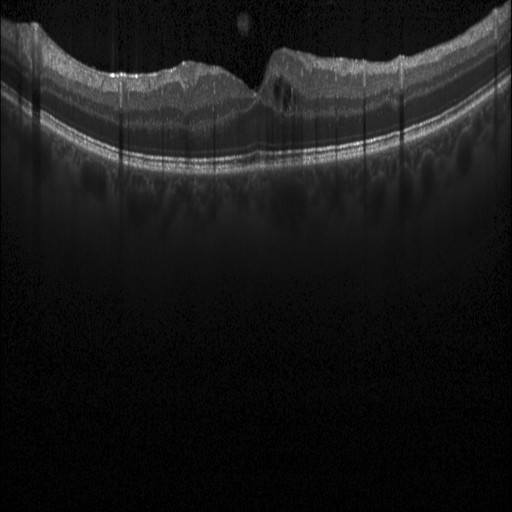 Retinal OCT cross-section. Acquired on a Heidelberg Spectralis.
Diabetic macular edema.